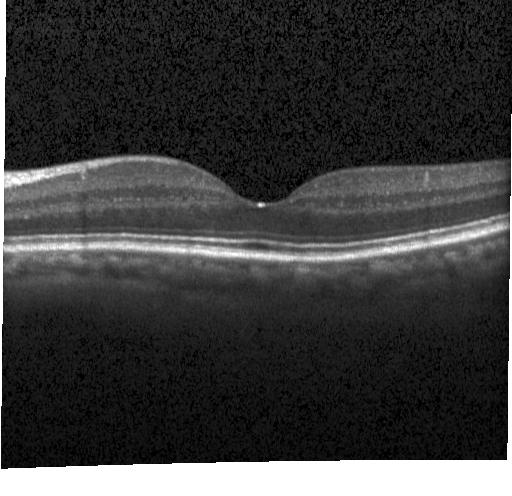 Horizontal scan through the fovea; acquired on a Heidelberg Spectralis; optical coherence tomography scan
Finding: no choroidal neovascularization, no diabetic macular edema, and no drusen.